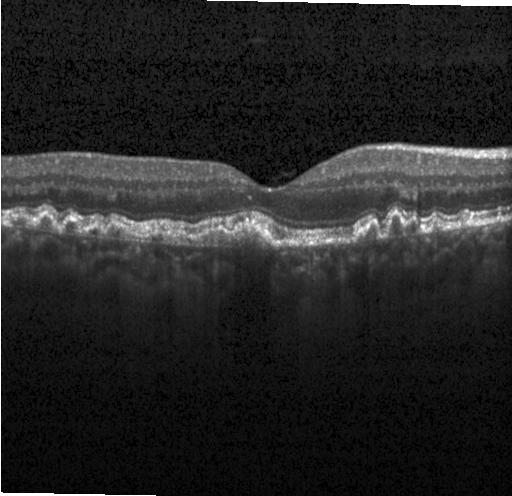 OCT line scan.
This B-scan demonstrates sub-RPE drusenoid deposits.